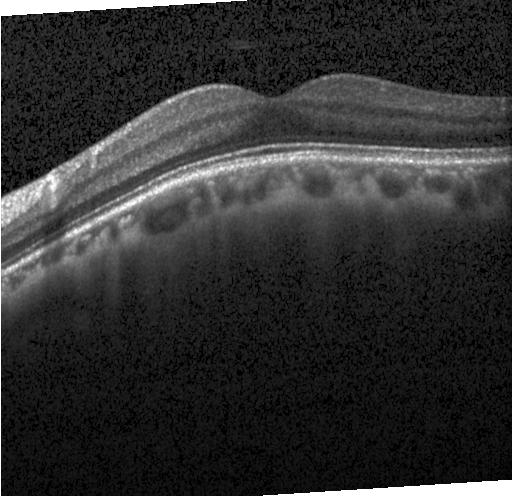 OCT B-scan · fovea-centered
Impression: neither choroidal neovascularization, diabetic macular edema, nor drusen.